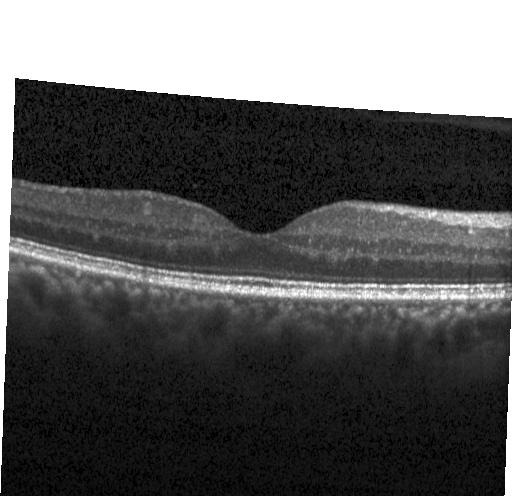

OCT B-scan; centered on the fovea.
Diagnosis: no CNV, DME, or drusen.